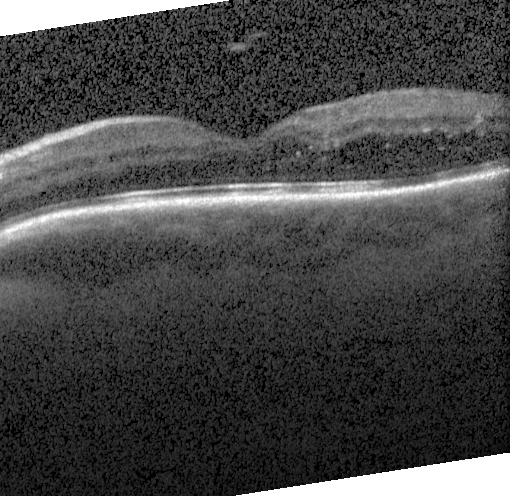

Finding: diabetic macular edema (DME).